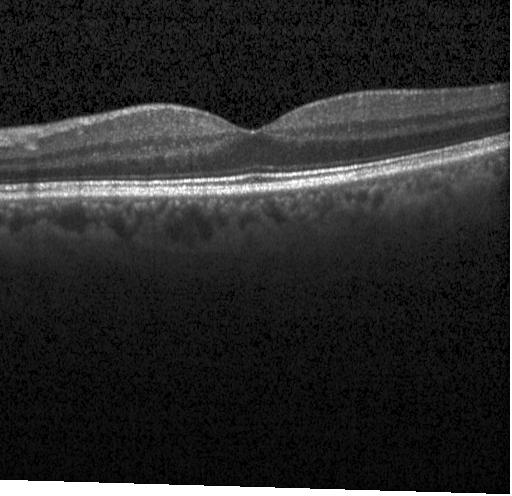 OCT B-scan; acquired on a Heidelberg Spectralis.
Impression: neither choroidal neovascularization, diabetic macular edema, nor drusen.